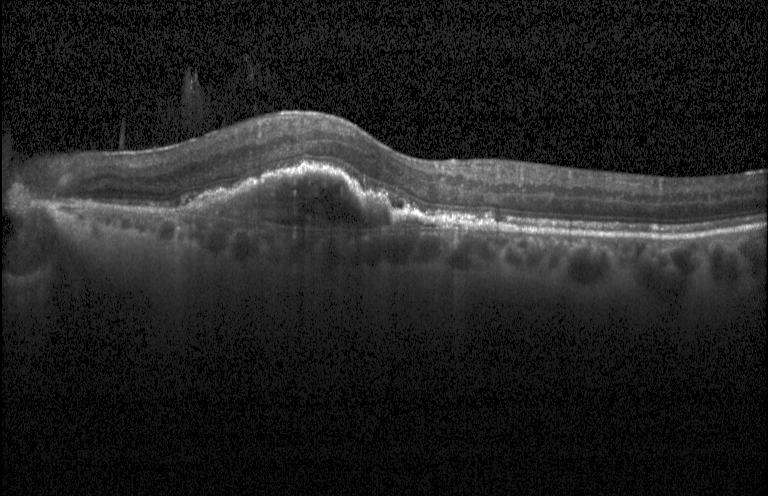
Diagnosis: choroidal neovascularization.